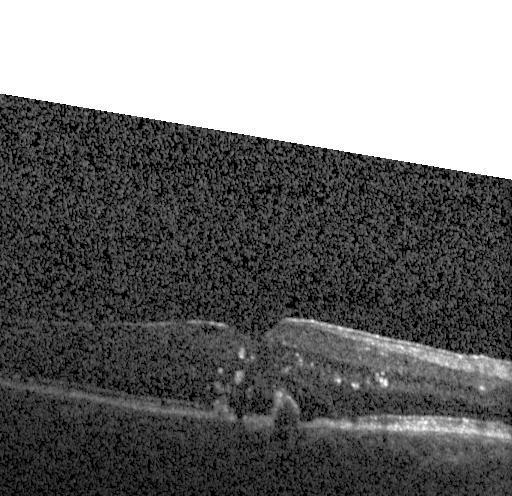

Optical coherence tomography B-scan. Impression: choroidal neovascularization.